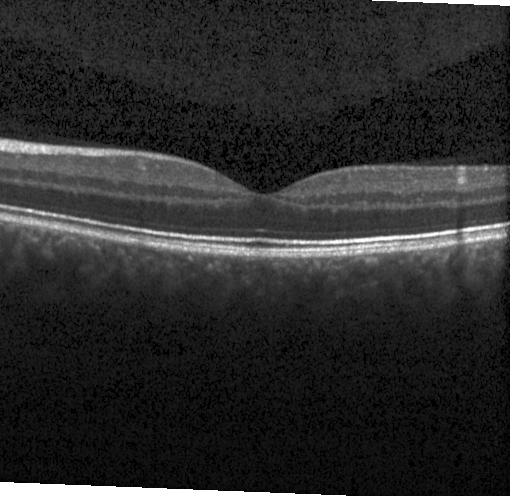
OCT finding: no choroidal neovascularization, diabetic macular edema, or drusen.